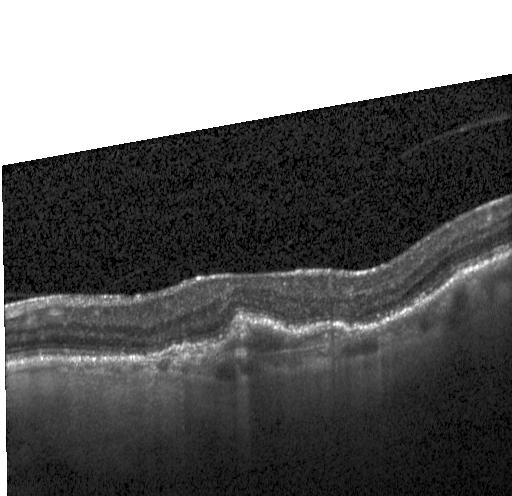 OCT line scan — The scan shows a choroidal neovascular membrane.